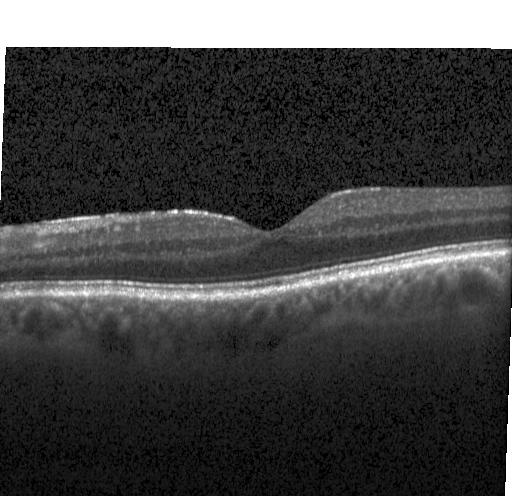 Retinal OCT cross-section, macular scan, spectral-domain OCT, acquired on a Heidelberg Spectralis — No evidence of CNV, DME, or drusen.